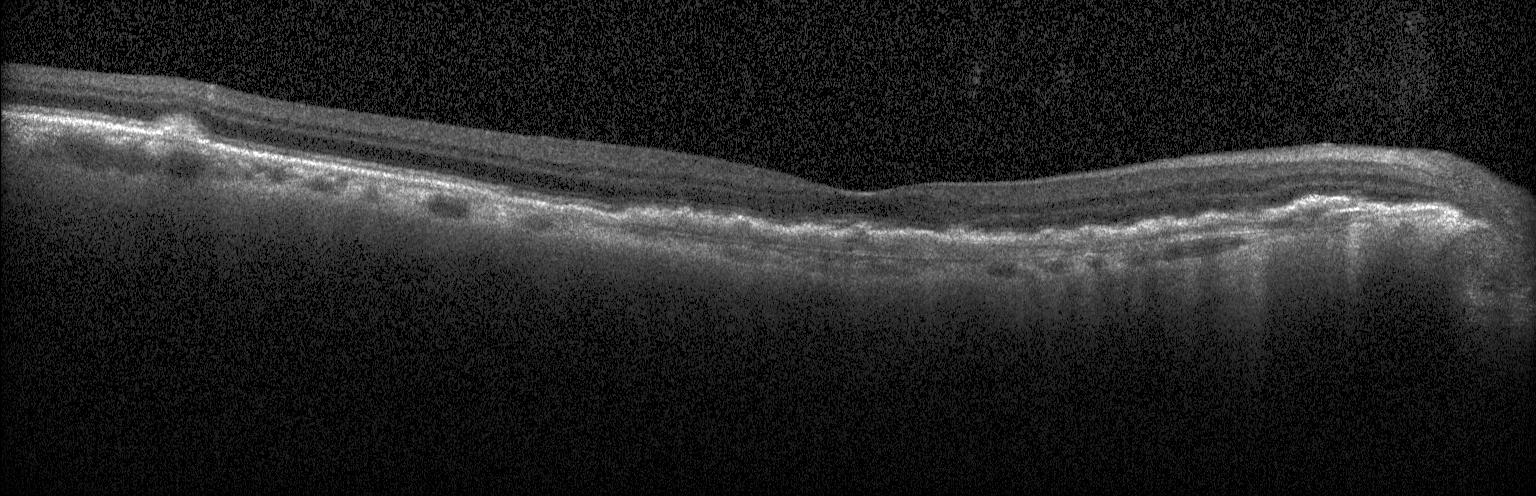
Centered on the fovea; OCT B-scan.
This B-scan demonstrates choroidal neovascularization.